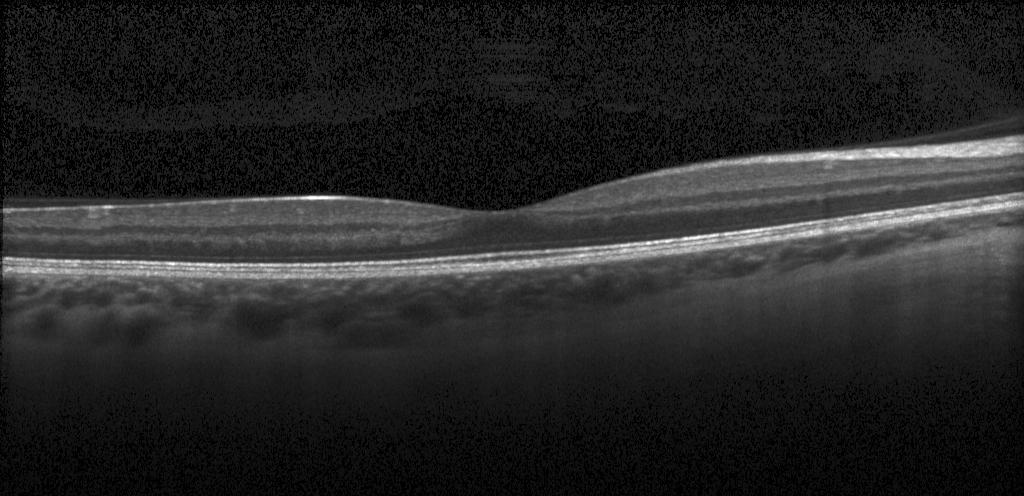 Retinal OCT cross-section; spectral-domain OCT. This B-scan demonstrates no choroidal neovascularization, no diabetic macular edema, and no drusen.